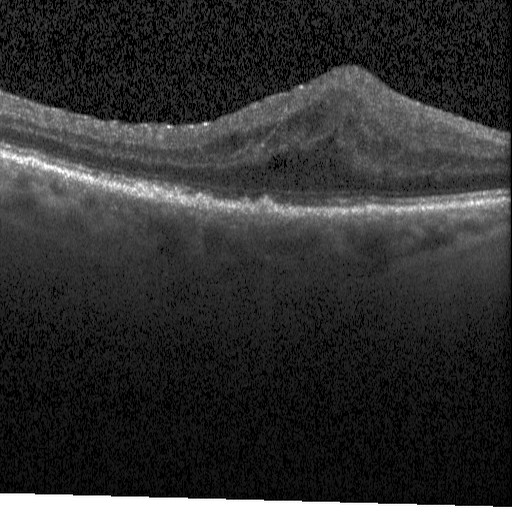
Heidelberg Spectralis OCT system; spectral-domain OCT; retinal OCT cross-section.
Impression: diabetic macular edema.